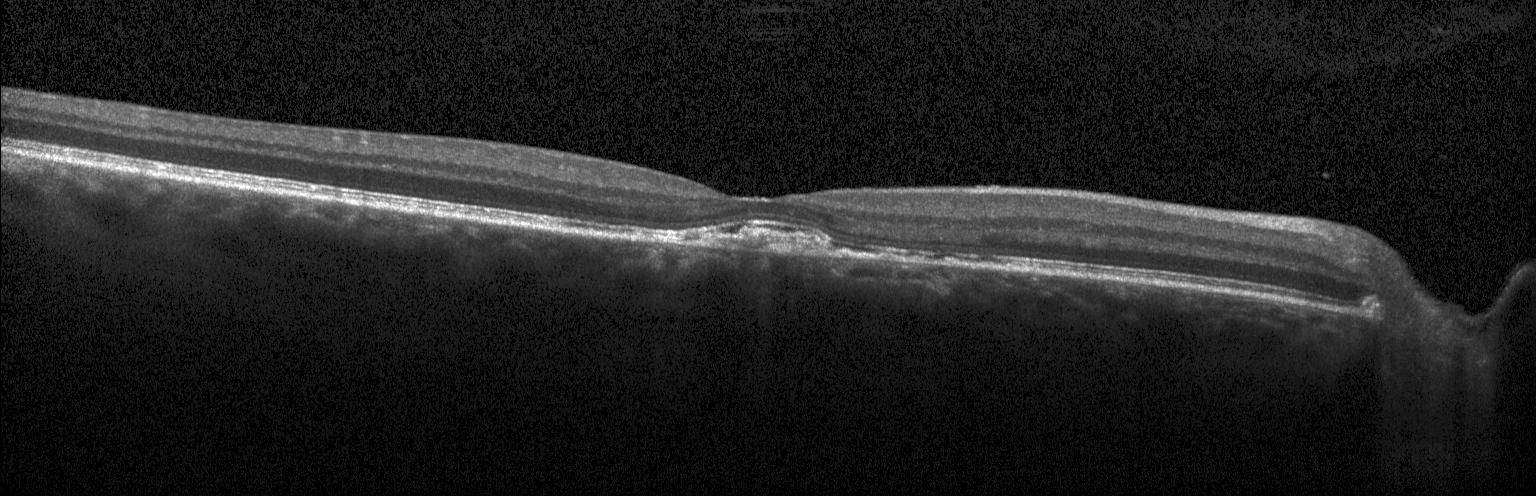 Finding: choroidal neovascularization.